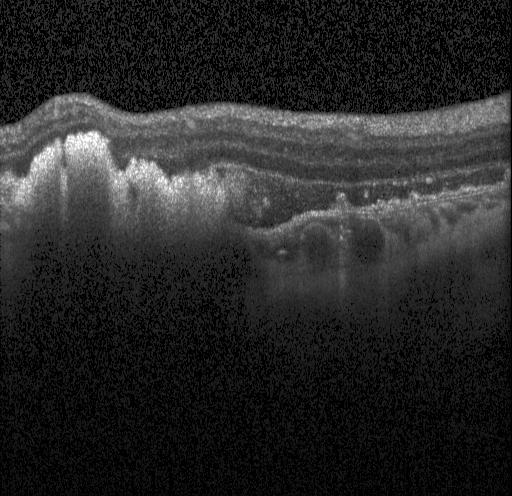

Finding: choroidal neovascularization (CNV).